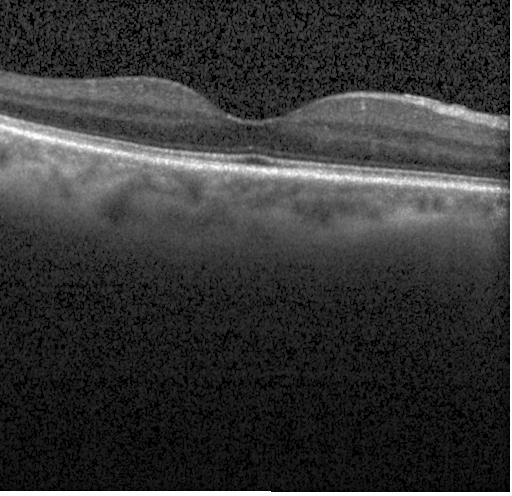
Impression: no choroidal neovascularization, no diabetic macular edema, and no drusen.